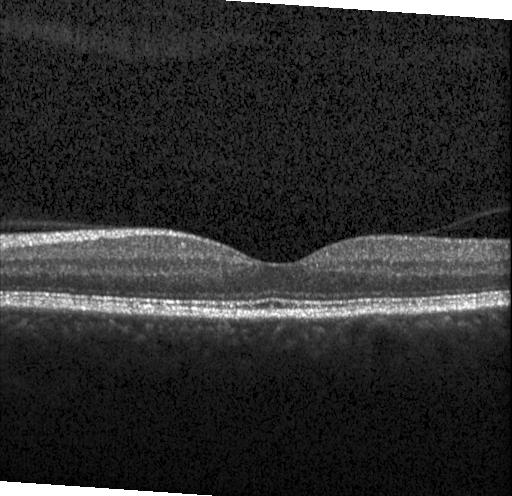 No evidence of choroidal neovascularization, diabetic macular edema, or drusen.